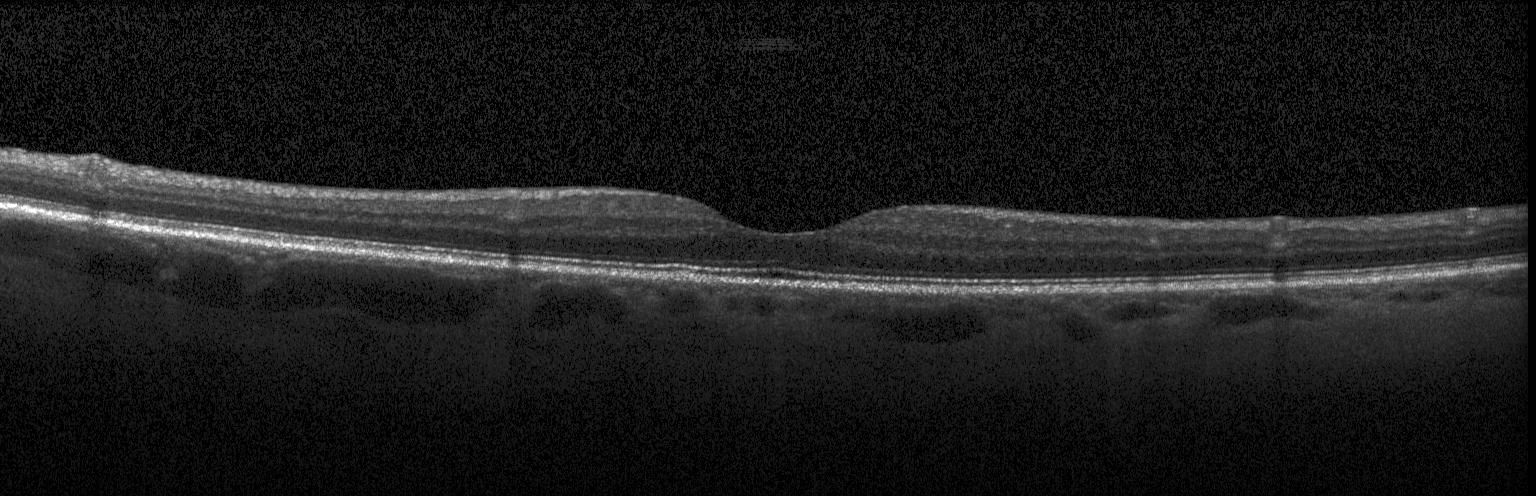
SD-OCT · OCT B-scan · through the macula · Heidelberg Spectralis
This B-scan demonstrates neither CNV, DME, nor drusen.